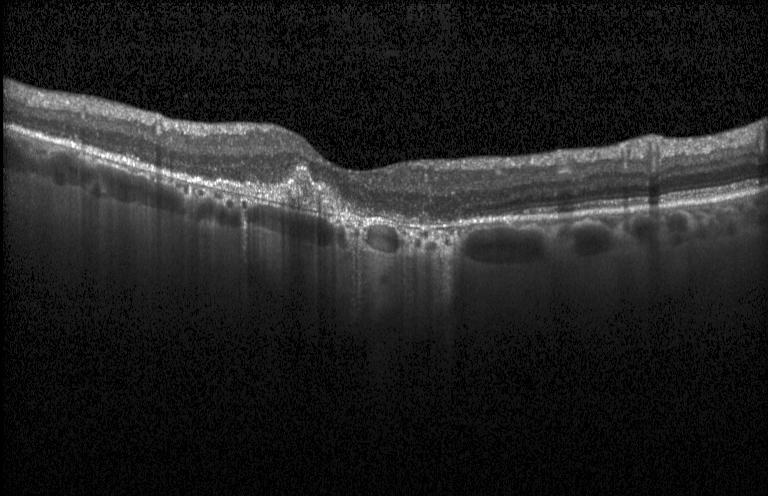

Instrument: Heidelberg Spectralis. OCT line scan.
Diagnosis: CNV.